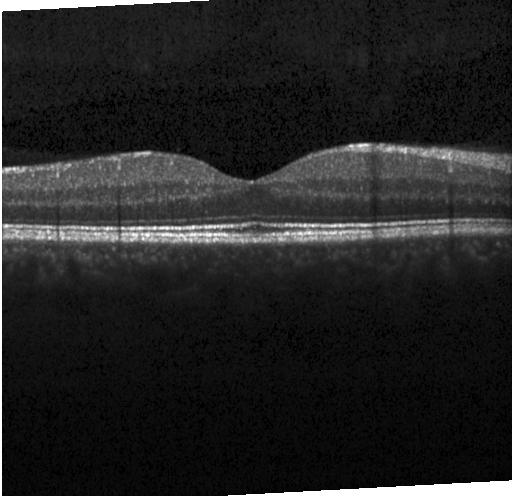
OCT scan showing no CNV, DME, or drusen.